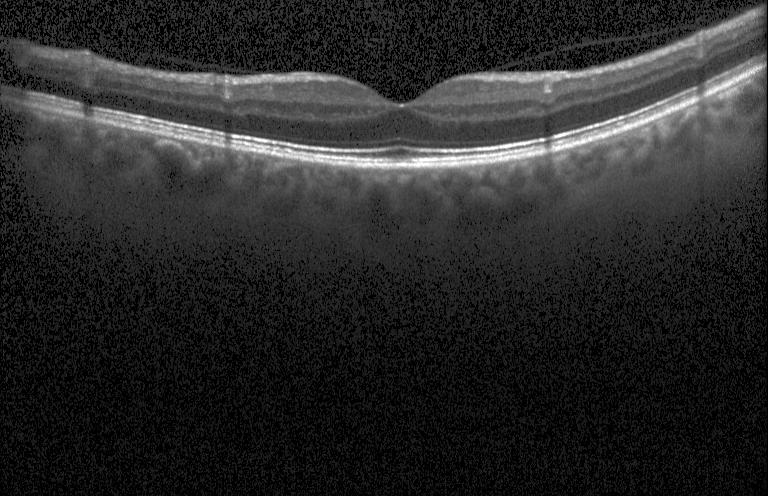
Impression: no evidence of choroidal neovascularization, diabetic macular edema, or drusen.